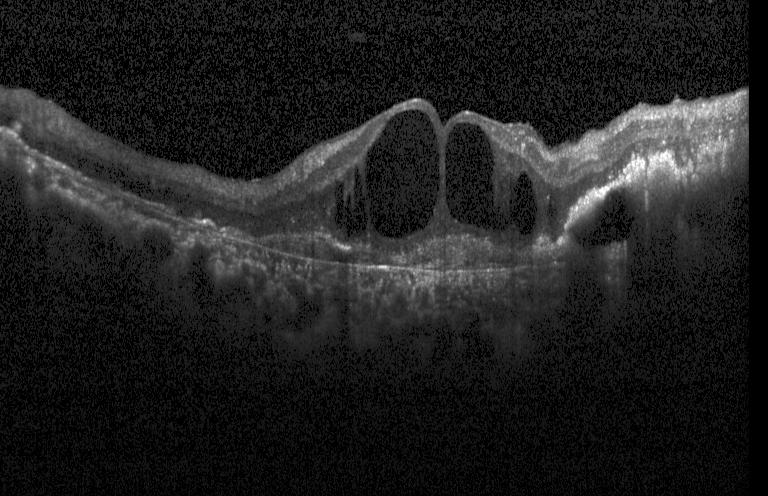

Spectral-domain OCT · OCT B-scan · macular scan · Heidelberg Spectralis — Finding: a choroidal neovascular membrane.